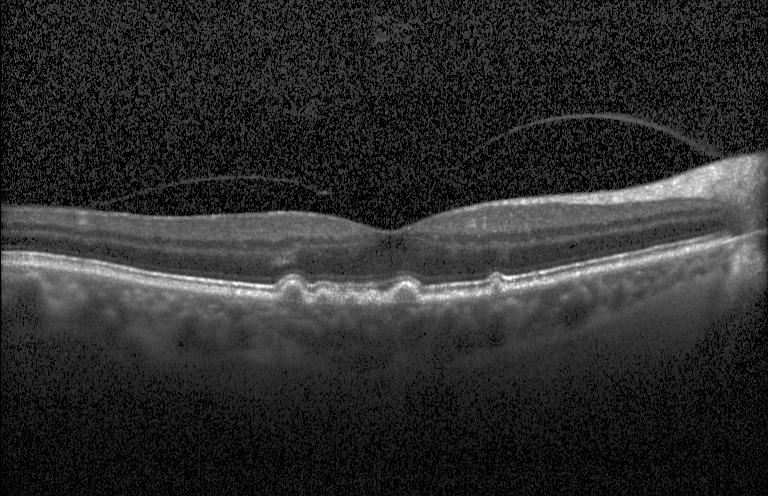
Retinal OCT cross-section
This B-scan demonstrates drusen.